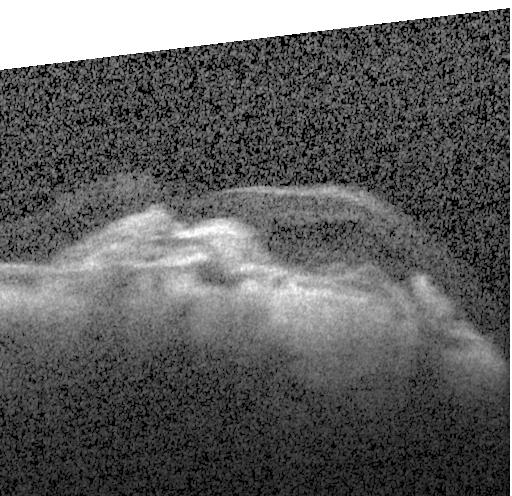 Retinal OCT B-scan. Fovea-centered. Spectral-domain OCT. Acquired on a Heidelberg Spectralis
Finding: CNV.